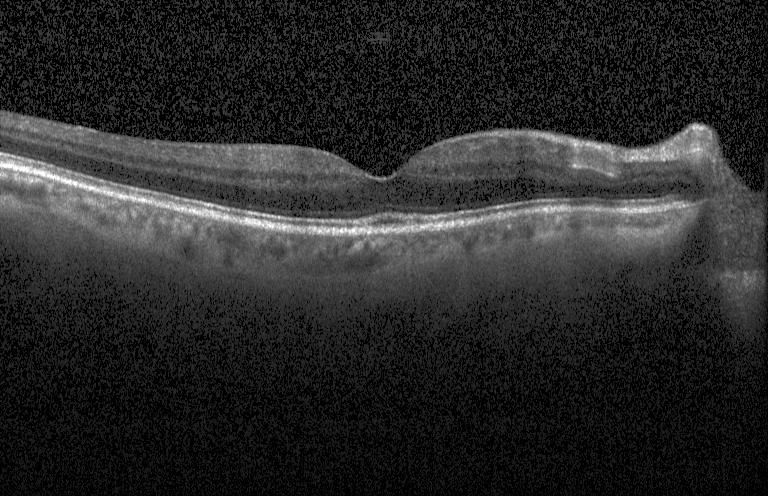
Finding: no evidence of CNV, DME, or drusen.